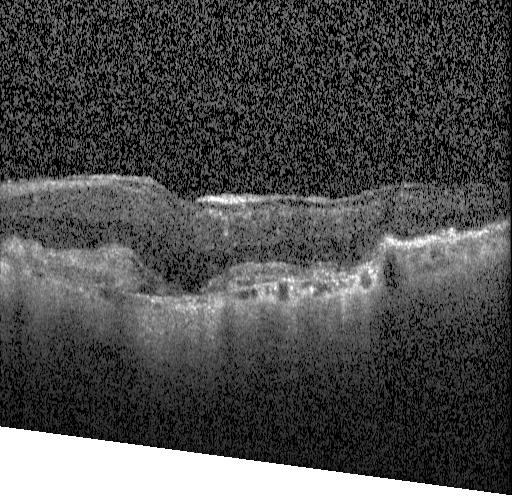 Retinal OCT B-scan. SD-OCT. Horizontal scan through the fovea. Finding: CNV.